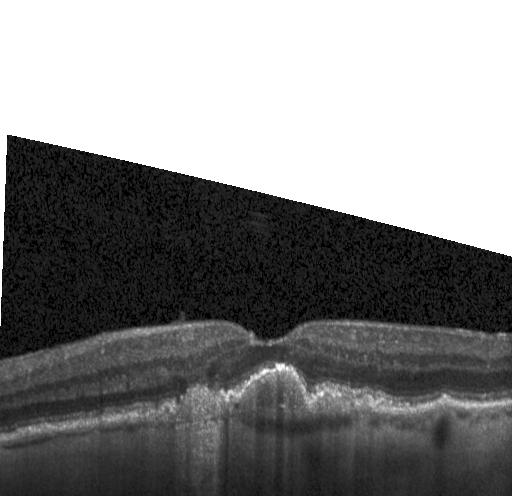
OCT finding: a choroidal neovascular membrane.